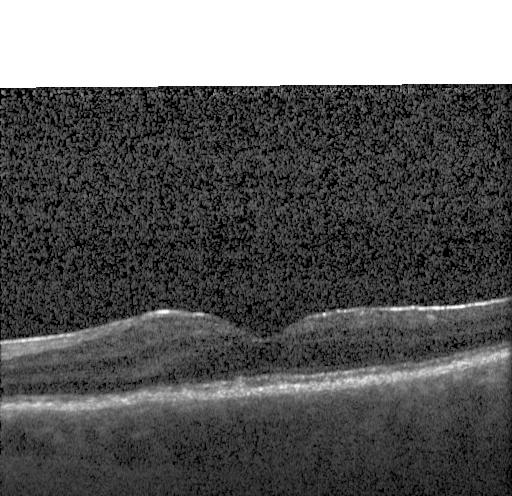

Retinal OCT cross-section showing neither choroidal neovascularization, diabetic macular edema, nor drusen.